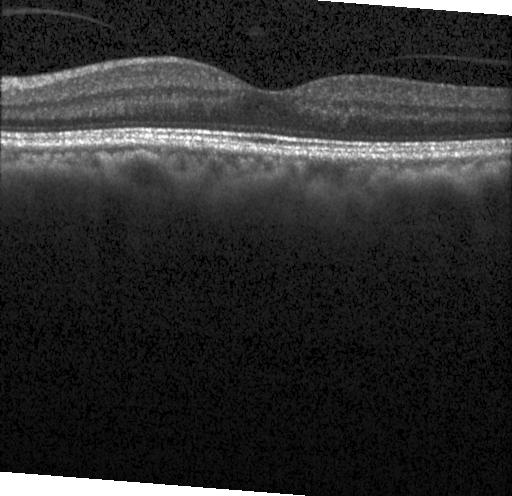 Retinal OCT cross-section; horizontal scan through the fovea
Diagnosis: neither choroidal neovascularization, diabetic macular edema, nor drusen.